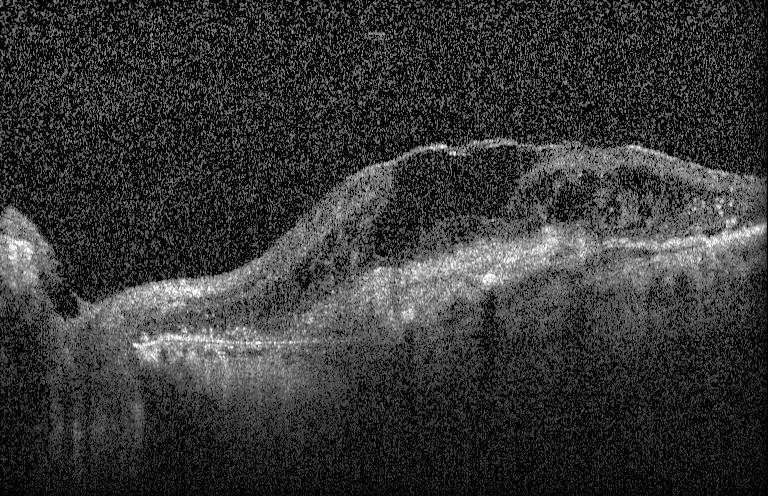 Finding: a choroidal neovascular membrane.